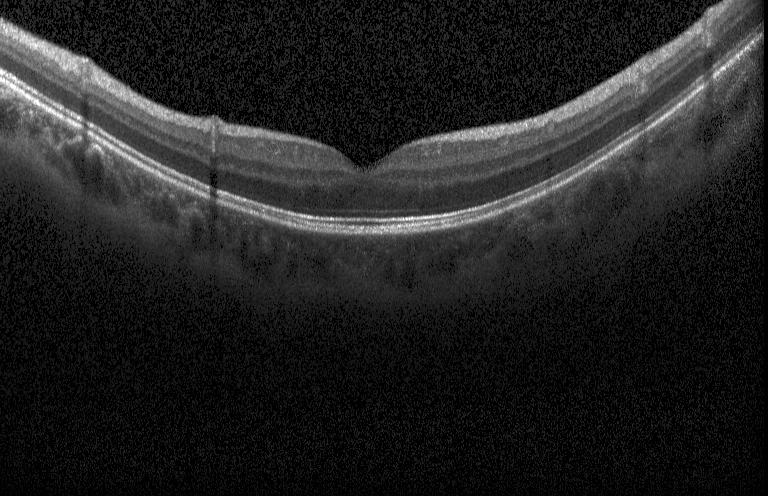
Macular OCT: neither CNV, DME, nor drusen.